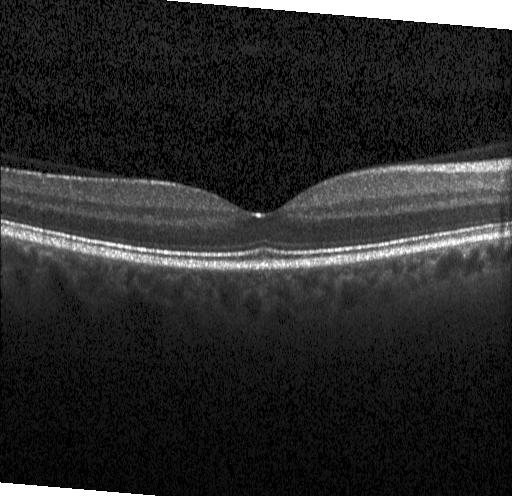

OCT line scan, centered on the fovea, spectral-domain OCT — Finding: no choroidal neovascularization, diabetic macular edema, or drusen.